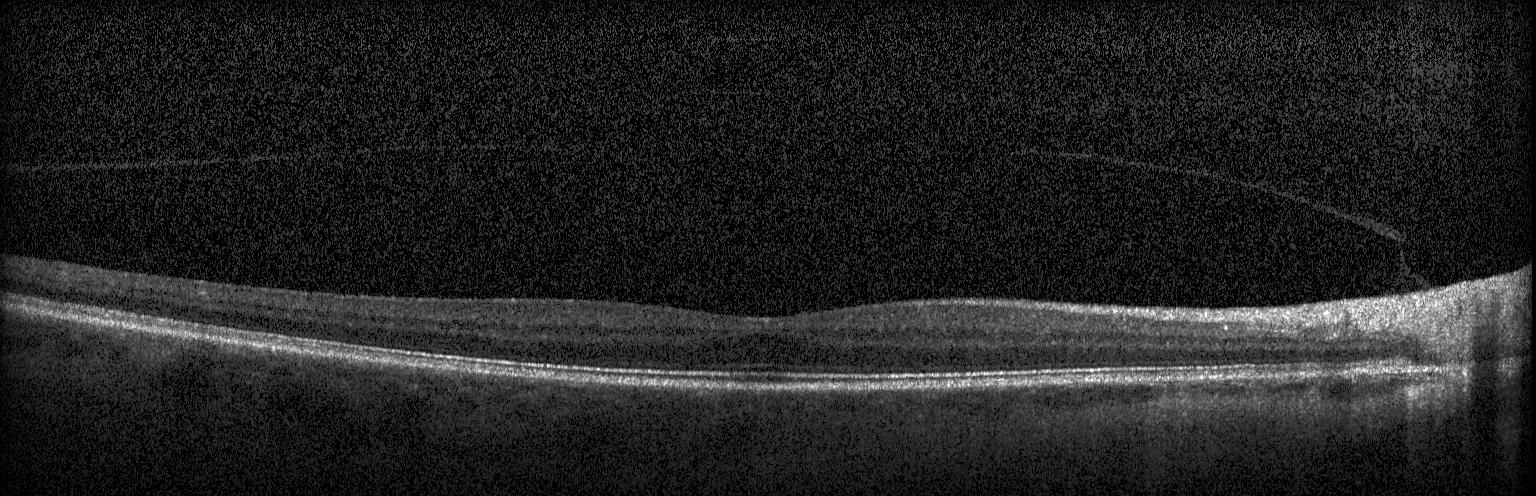

Heidelberg Spectralis · optical coherence tomography scan — Dx: no evidence of choroidal neovascularization, diabetic macular edema, or drusen.